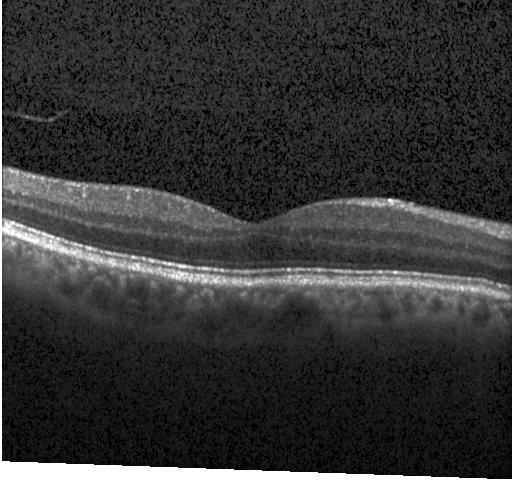
Impression: no evidence of choroidal neovascularization, diabetic macular edema, or drusen.